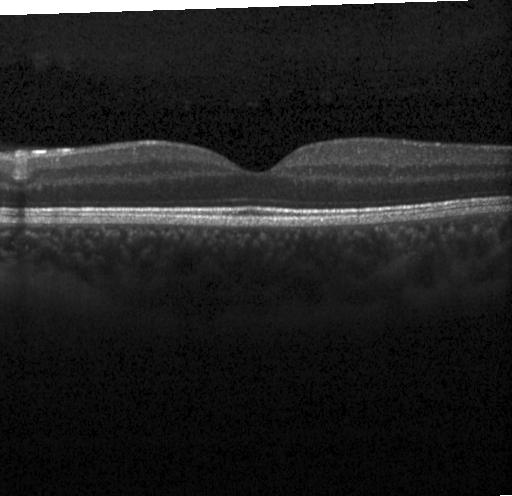 Heidelberg Spectralis, spectral-domain optical coherence tomography, horizontal scan through the fovea, optical coherence tomography B-scan
Macular OCT: neither choroidal neovascularization, diabetic macular edema, nor drusen.